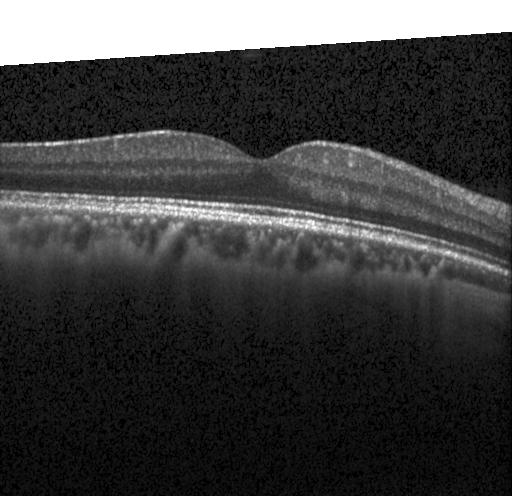

Optical coherence tomography B-scan, Heidelberg Spectralis OCT system, macular scan. Dx: no choroidal neovascularization, no diabetic macular edema, and no drusen.